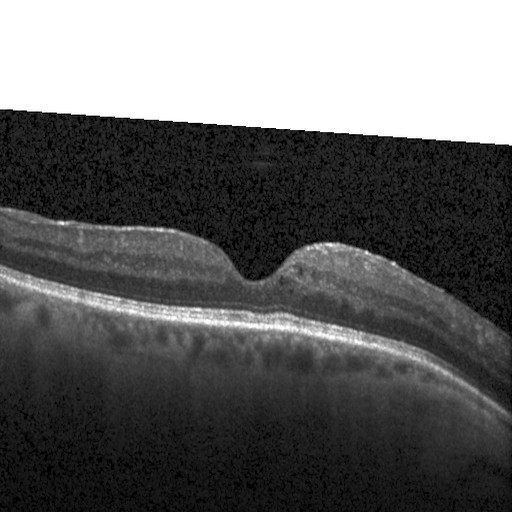 Retinal OCT cross-section — Dx: diabetic macular edema.